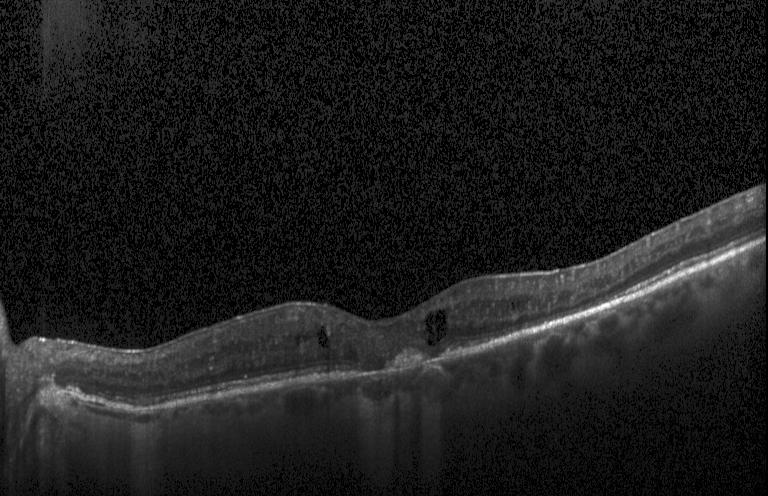
This B-scan demonstrates a choroidal neovascular membrane.